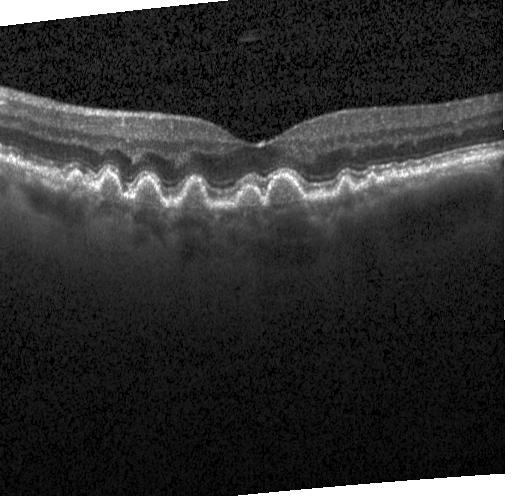

Impression: sub-RPE drusenoid deposits.